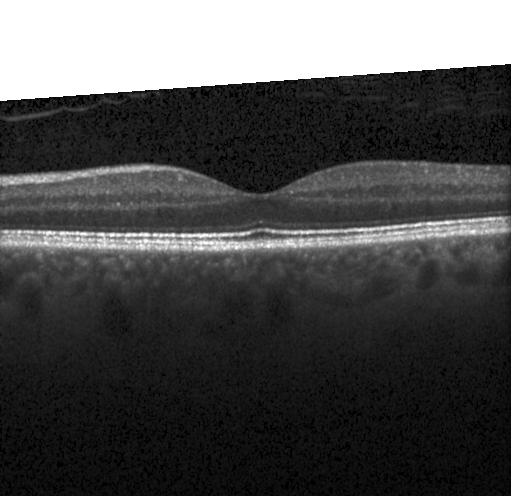

Impression: no CNV, DME, or drusen.